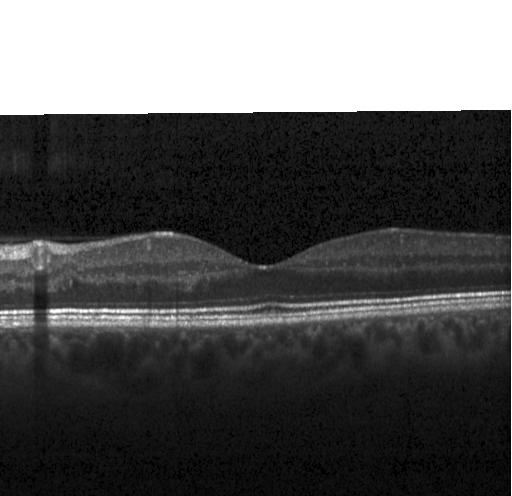

Acquired on a Heidelberg Spectralis. Through the macula. Optical coherence tomography scan. Diagnosis: neither CNV, DME, nor drusen.